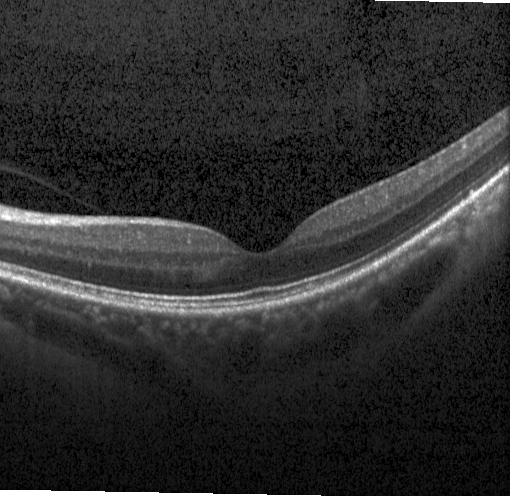 Macular OCT demonstrating no CNV, no DME, and no drusen.